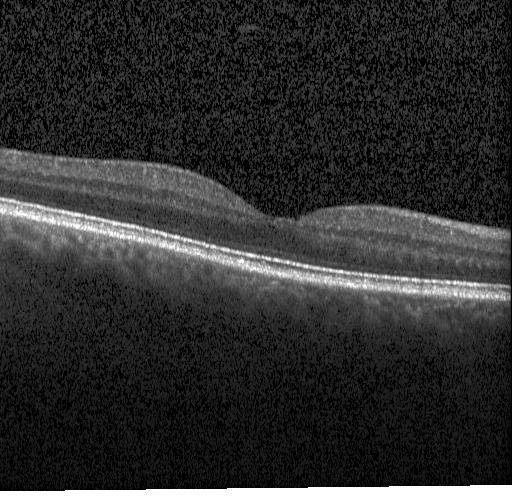

Heidelberg Spectralis. SD-OCT. Retinal OCT cross-section. Centered on the fovea.
Finding: neither choroidal neovascularization, diabetic macular edema, nor drusen.